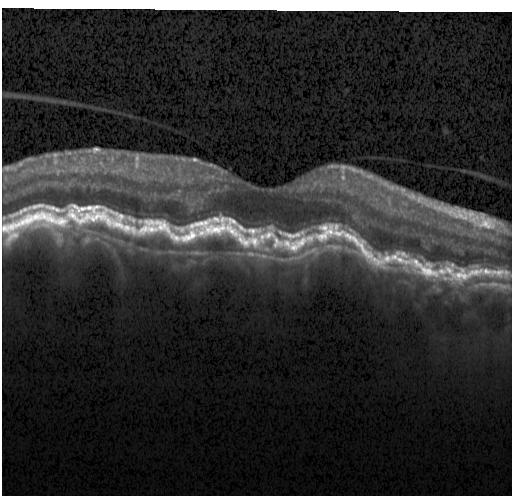

Optical coherence tomography B-scan. Finding: a choroidal neovascular membrane.